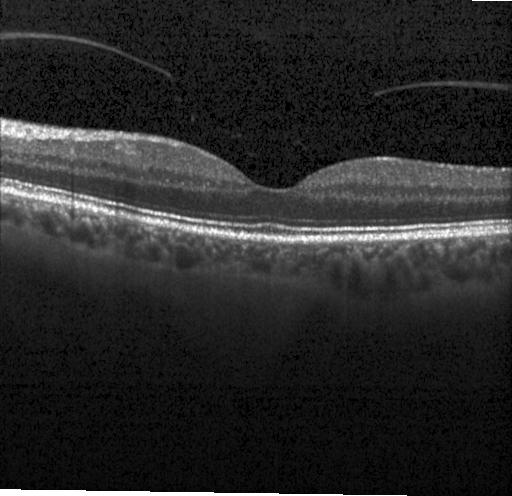
Macular OCT demonstrating no evidence of choroidal neovascularization, diabetic macular edema, or drusen.